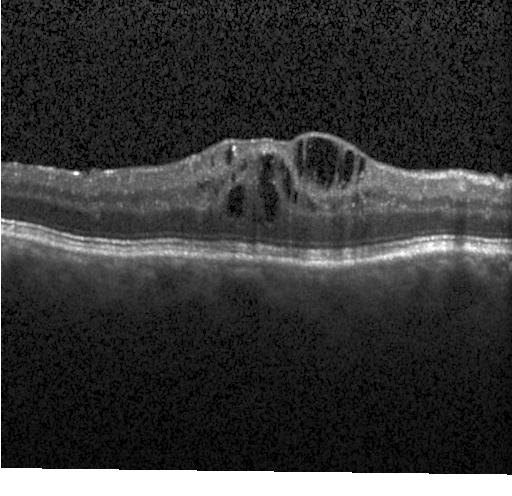

Diagnosis: diabetic macular edema.